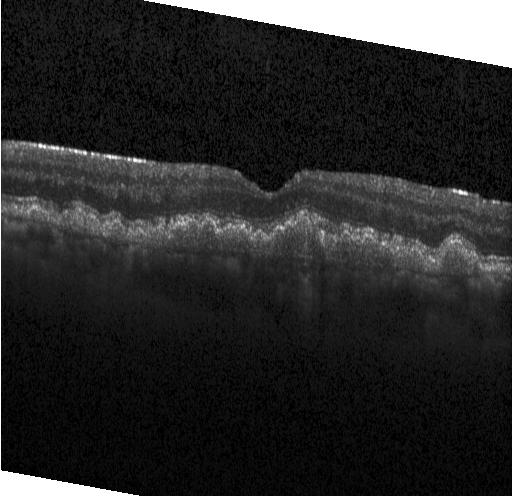
Spectral-domain optical coherence tomography, through the macula, optical coherence tomography B-scan, Heidelberg Spectralis OCT system — OCT finding: a choroidal neovascular membrane.